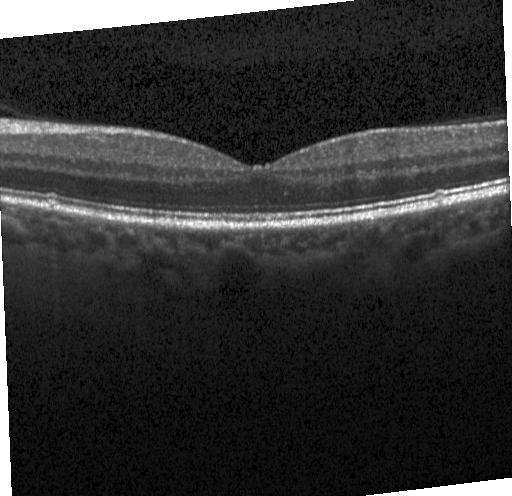 Optical coherence tomography scan, spectral-domain OCT, fovea-centered, instrument: Heidelberg Spectralis.
Impression: sub-RPE drusenoid deposits.